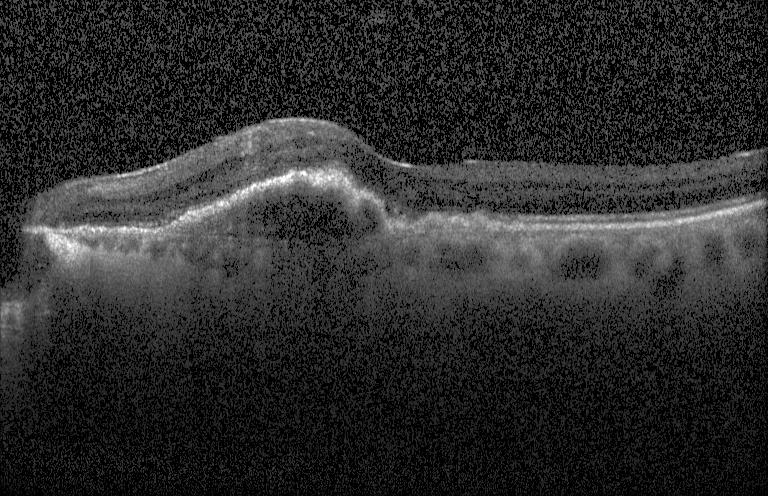

Macular OCT demonstrating a choroidal neovascular membrane.